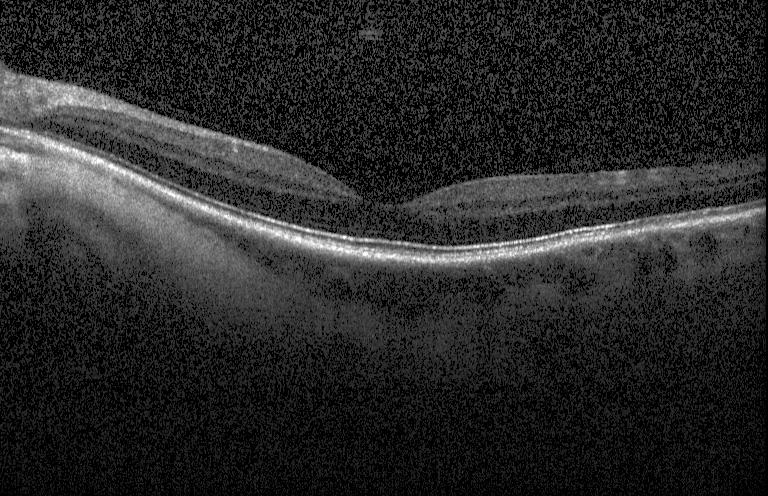
OCT finding: no evidence of choroidal neovascularization, diabetic macular edema, or drusen.